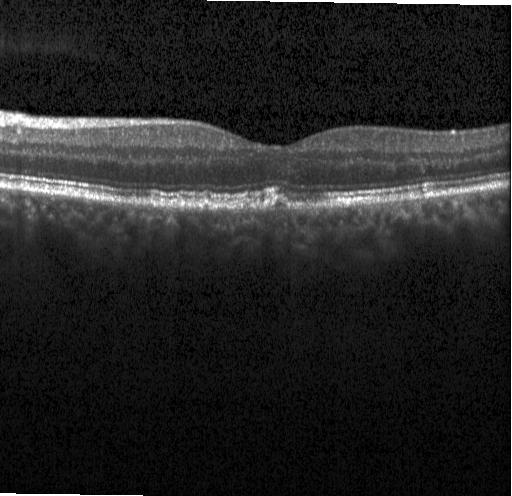 Dx: drusen.